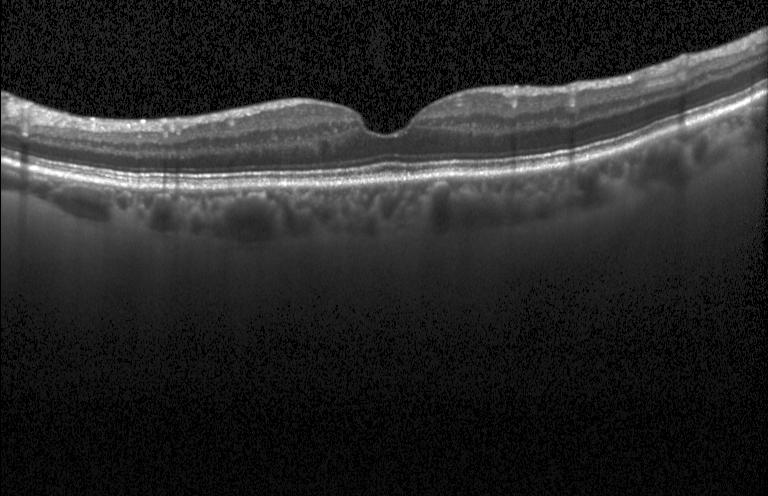

SD-OCT. Fovea-centered. Optical coherence tomography scan.
Finding: no choroidal neovascularization, diabetic macular edema, or drusen.